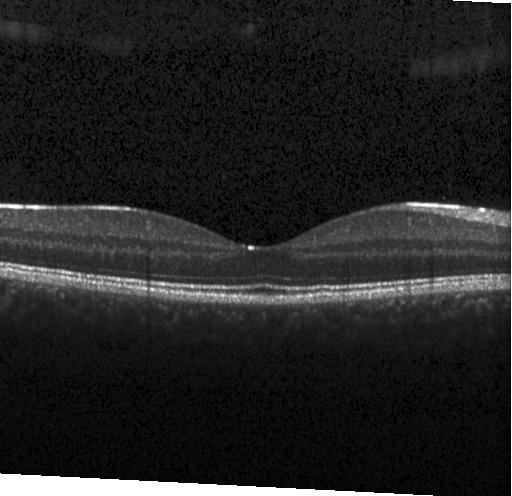

Acquired on a Heidelberg Spectralis; retinal OCT cross-section; fovea-centered. Finding: no CNV, no DME, and no drusen.